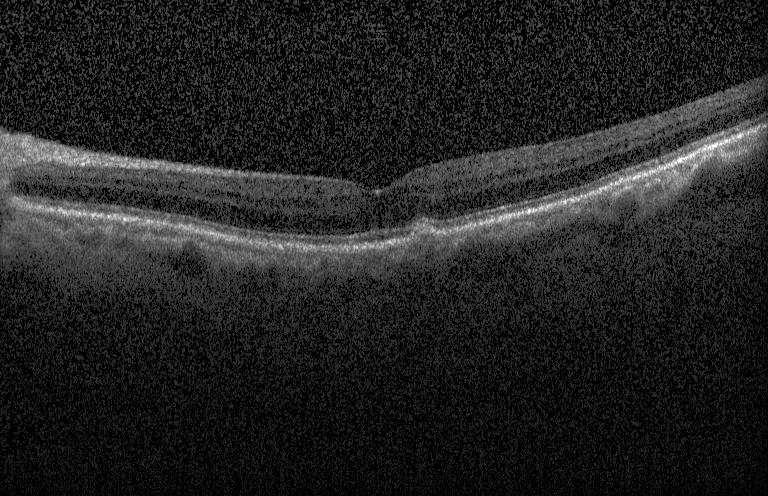
Instrument: Heidelberg Spectralis, SD-OCT, optical coherence tomography scan, horizontal scan through the fovea. Diagnosis: drusen.